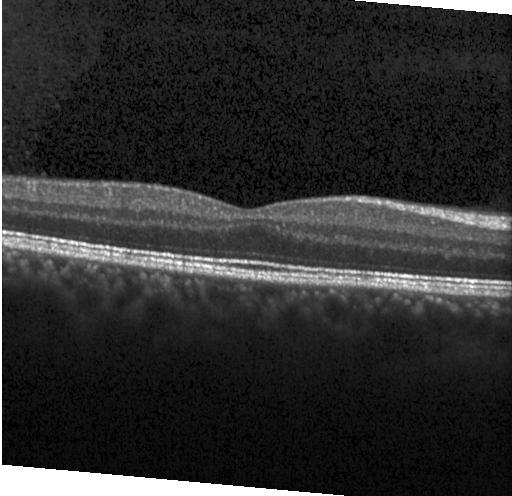

OCT line scan — The scan shows neither choroidal neovascularization, diabetic macular edema, nor drusen.